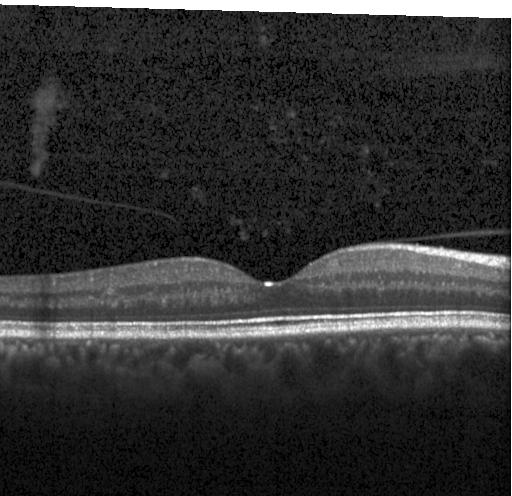

Heidelberg Spectralis; retinal OCT B-scan; spectral-domain optical coherence tomography
Dx: neither CNV, DME, nor drusen.